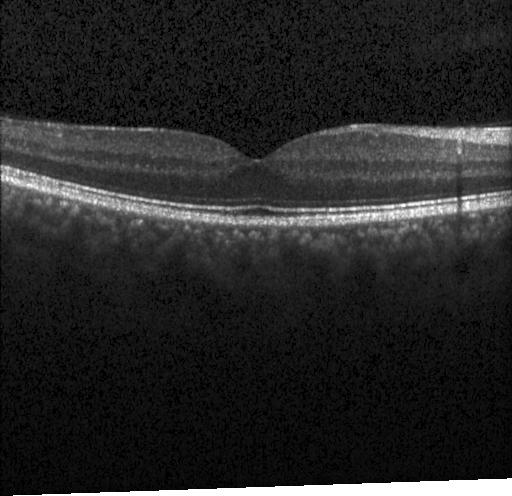
Spectral-domain OCT B-scan: no CNV, no DME, and no drusen.